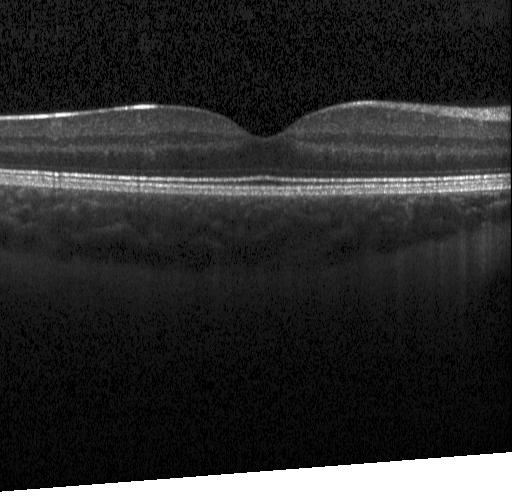 Spectral-domain OCT; retinal OCT cross-section; macular scan — Impression: neither CNV, DME, nor drusen.